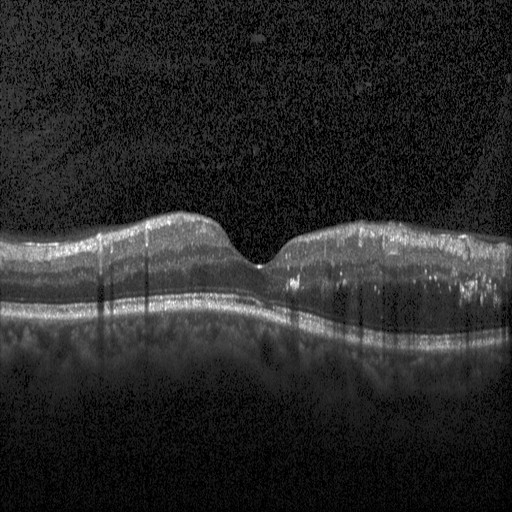

Retinal OCT cross-section, spectral-domain optical coherence tomography, instrument: Heidelberg Spectralis.
This B-scan demonstrates DME.